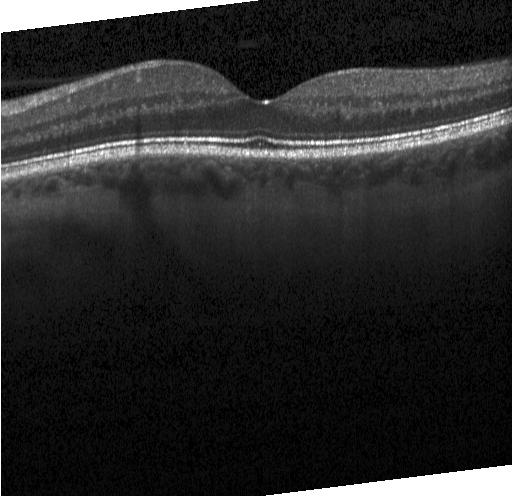
OCT B-scan.
Macular OCT: no CNV, no DME, and no drusen.